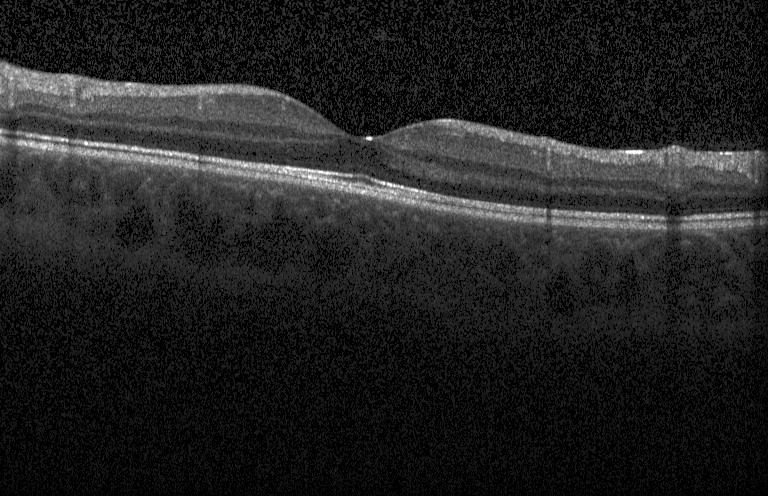
OCT line scan · centered on the fovea · spectral-domain OCT.
OCT finding: no evidence of CNV, DME, or drusen.